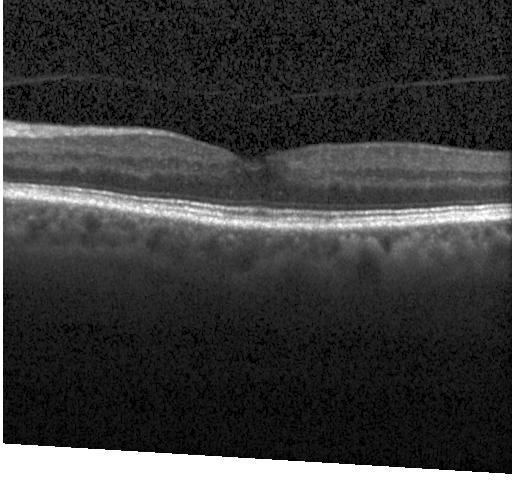
Spectral-domain optical coherence tomography, macular scan, retinal OCT B-scan, acquired on a Heidelberg Spectralis — Macular OCT: no CNV, DME, or drusen.